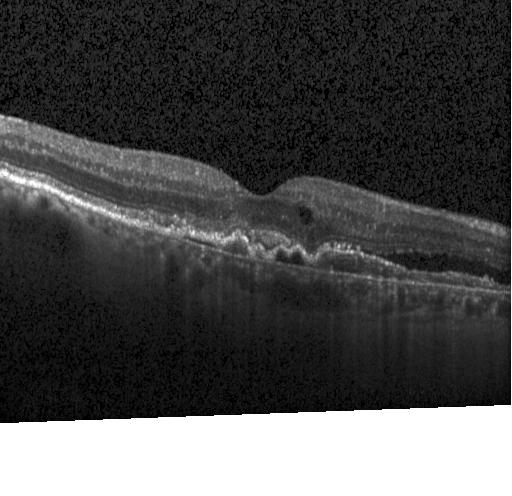
OCT scan showing choroidal neovascularization (CNV).